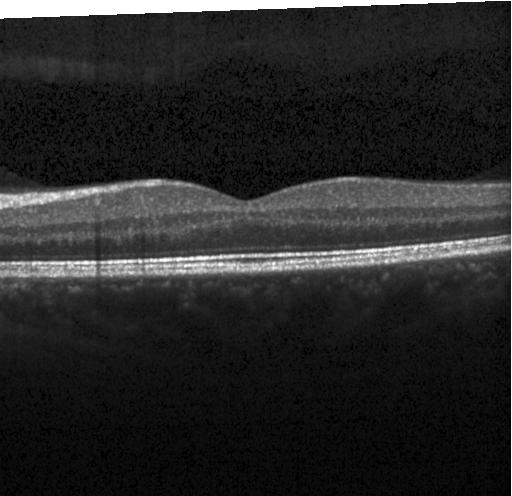
Assessment: neither choroidal neovascularization, diabetic macular edema, nor drusen.